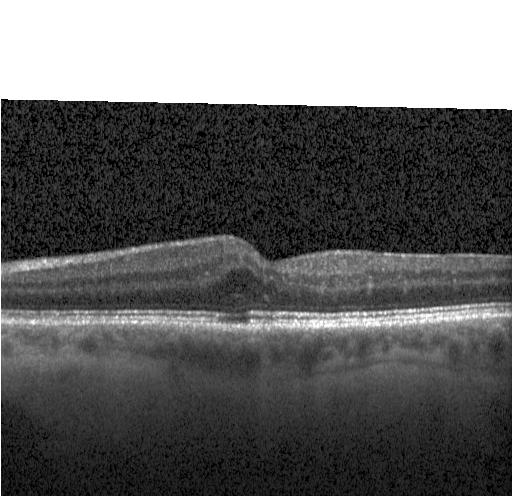

Spectral-domain optical coherence tomography. Heidelberg Spectralis OCT system. OCT line scan
This B-scan demonstrates diabetic macular edema.